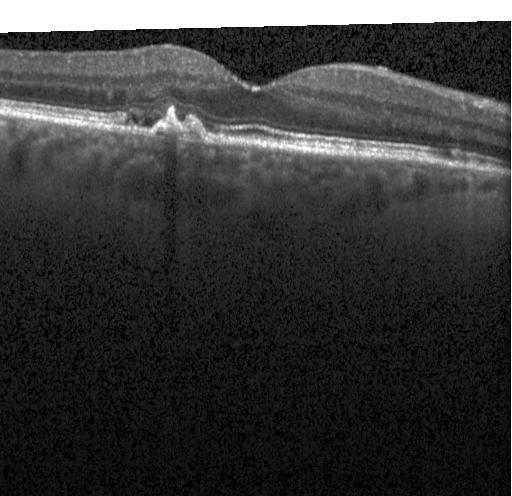 Spectral-domain OCT · OCT B-scan · acquired on a Heidelberg Spectralis · through the macula
Diagnosis: CNV.